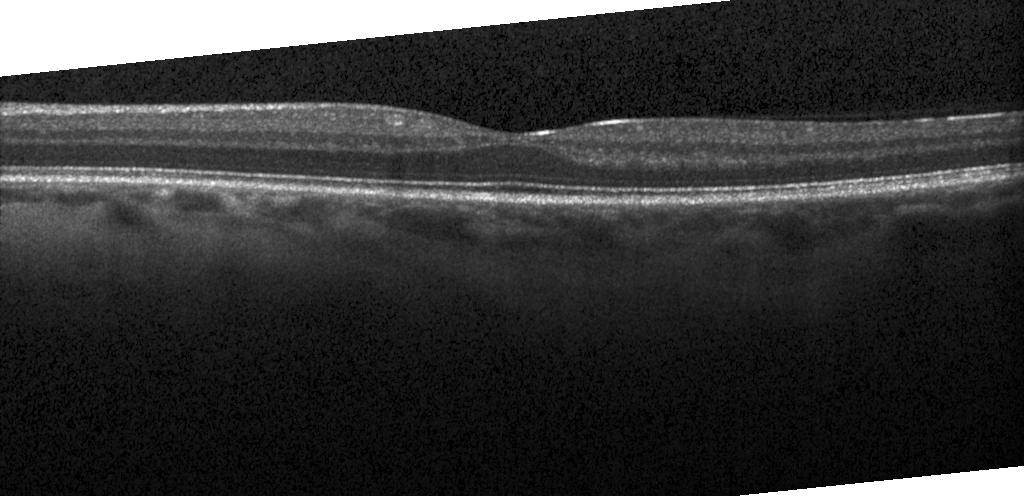 Fovea-centered · optical coherence tomography B-scan — This B-scan demonstrates no evidence of CNV, DME, or drusen.